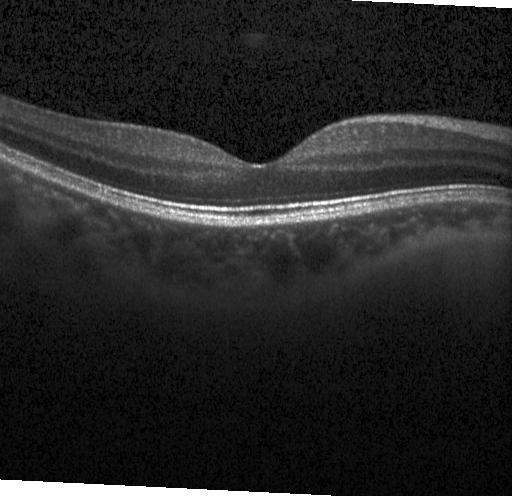

Optical coherence tomography B-scan.
No CNV, DME, or drusen.